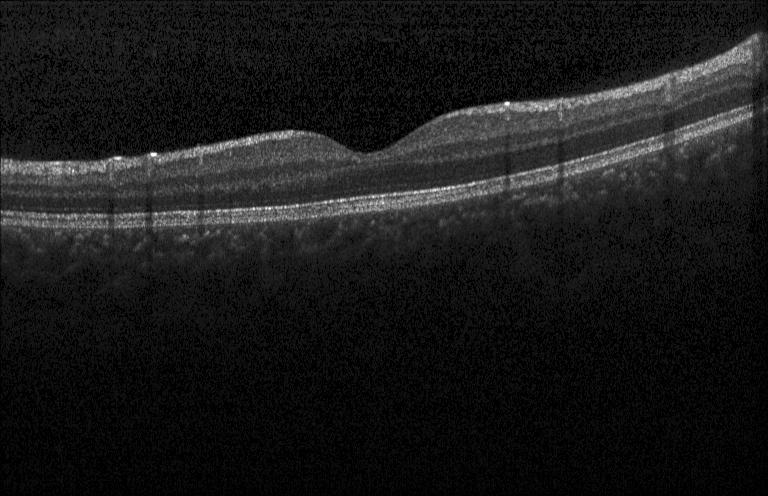 No choroidal neovascularization, diabetic macular edema, or drusen.